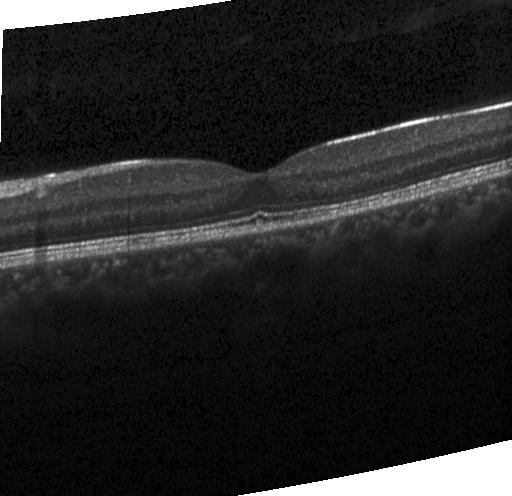
Spectral-domain OCT. Retinal OCT cross-section. Instrument: Heidelberg Spectralis
Diagnosis: no choroidal neovascularization, no diabetic macular edema, and no drusen.